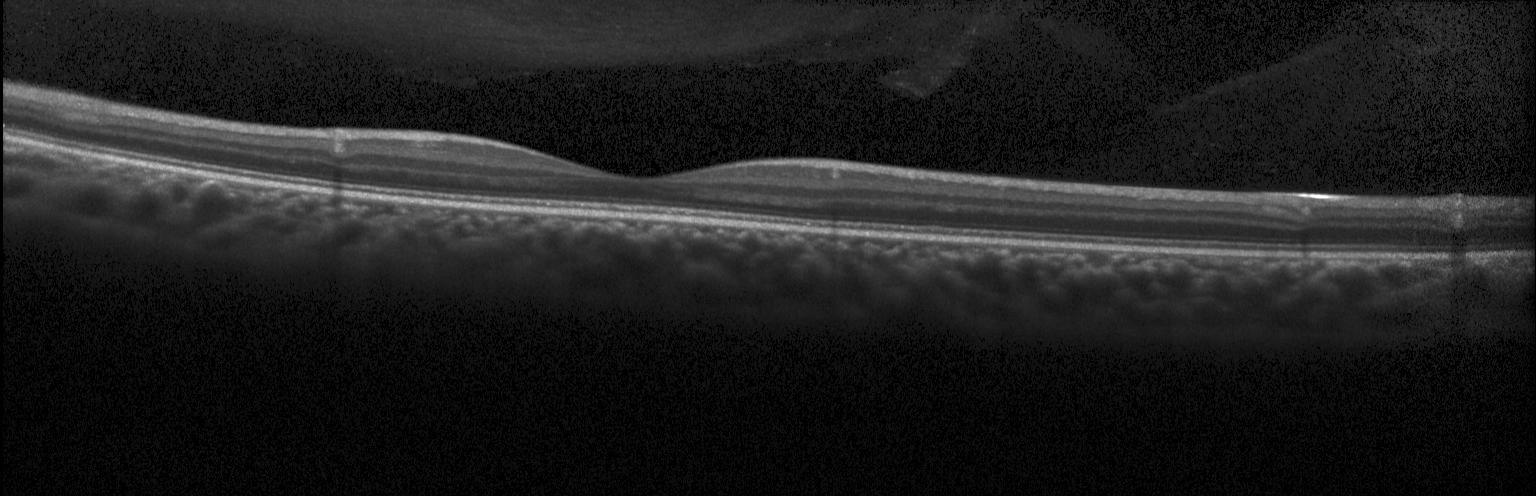 Finding: no choroidal neovascularization, diabetic macular edema, or drusen.